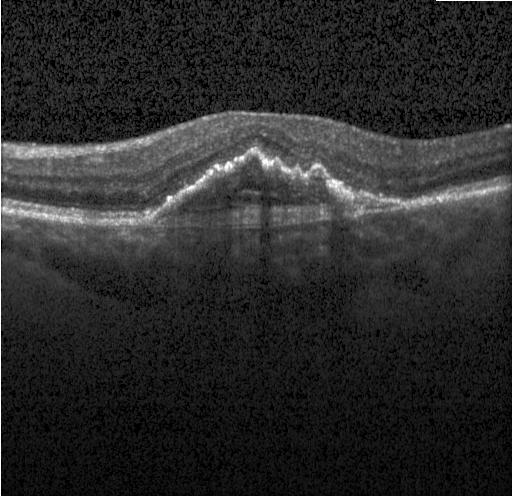 Horizontal scan through the fovea · Heidelberg Spectralis · optical coherence tomography scan — Impression: choroidal neovascularization (CNV).